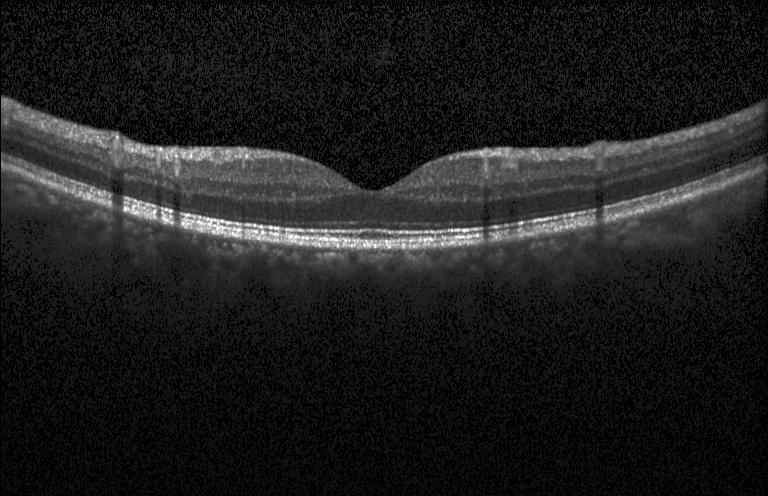

SD-OCT; retinal OCT B-scan; Heidelberg Spectralis OCT system
Diagnosis: neither CNV, DME, nor drusen.